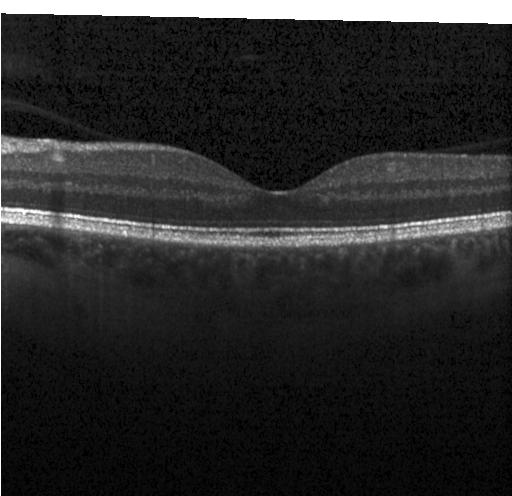
Optical coherence tomography B-scan · horizontal scan through the fovea
Diagnosis: no evidence of choroidal neovascularization, diabetic macular edema, or drusen.